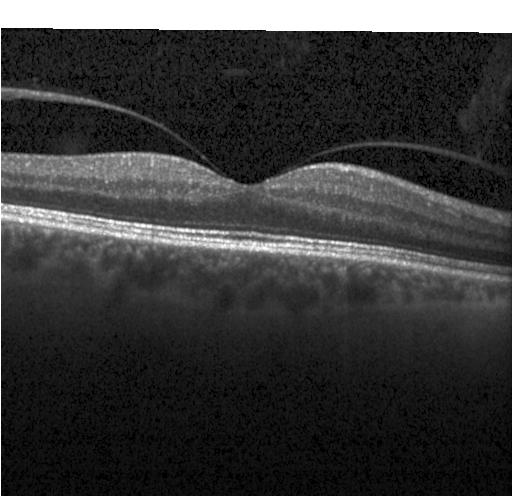
Retinal OCT cross-section. Horizontal scan through the fovea. This B-scan demonstrates neither CNV, DME, nor drusen.